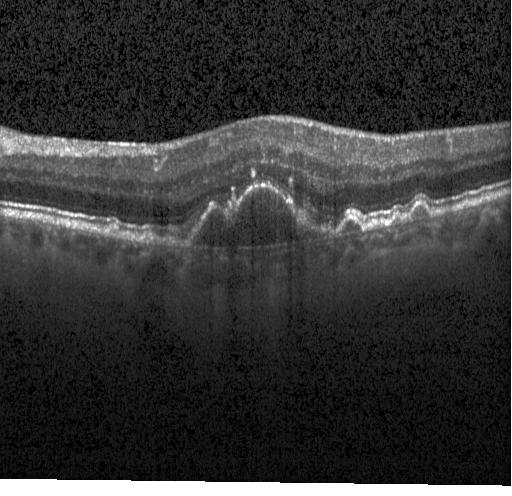

Optical coherence tomography scan; centered on the fovea. The scan shows choroidal neovascularization.